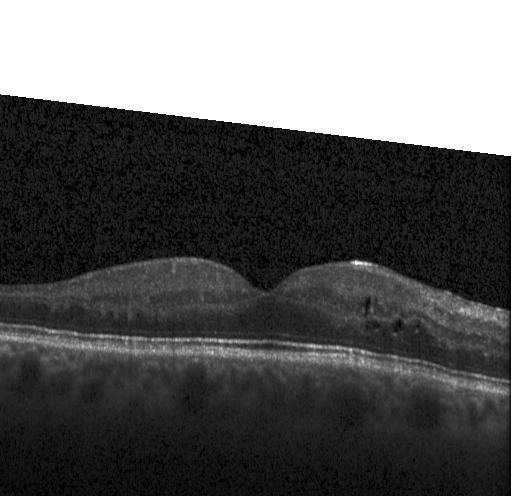 Diagnosis: DME.